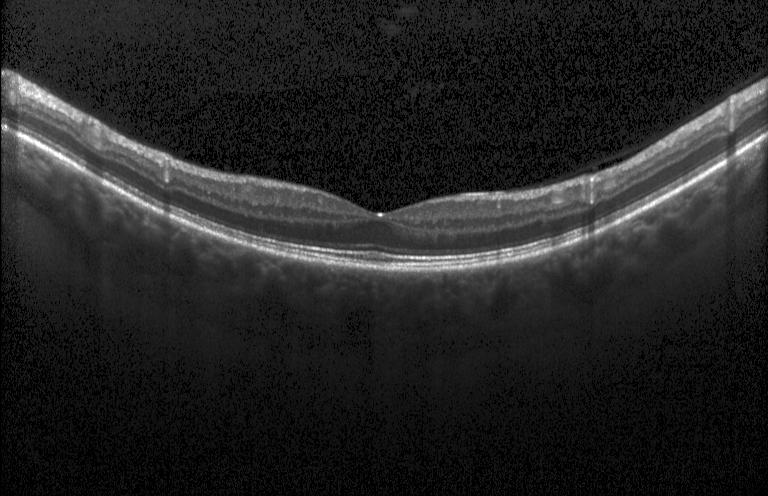

Impression: no evidence of CNV, DME, or drusen.